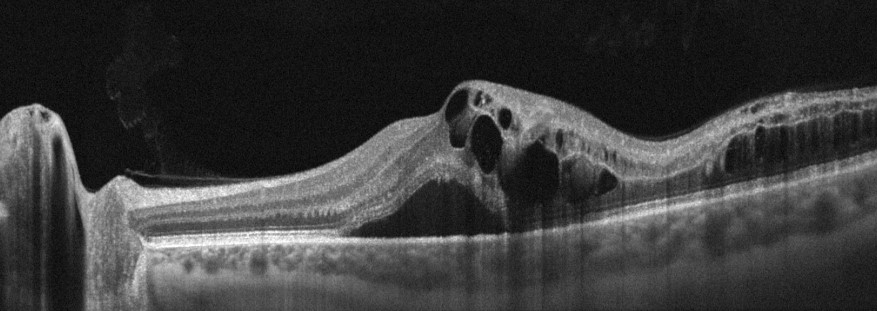
OCT line scan.
The scan shows RVO.